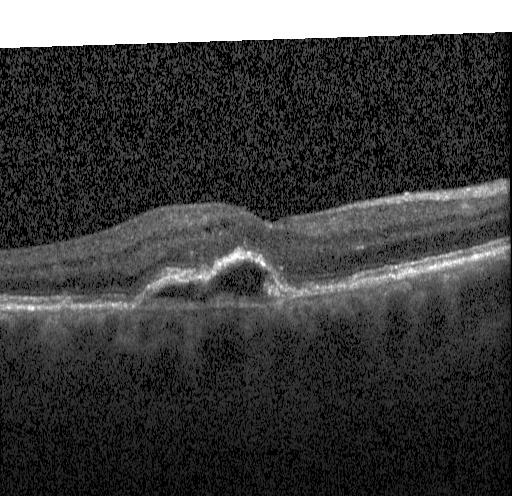

Retinal OCT cross-section, spectral-domain OCT, horizontal scan through the fovea. Finding: a choroidal neovascular membrane.